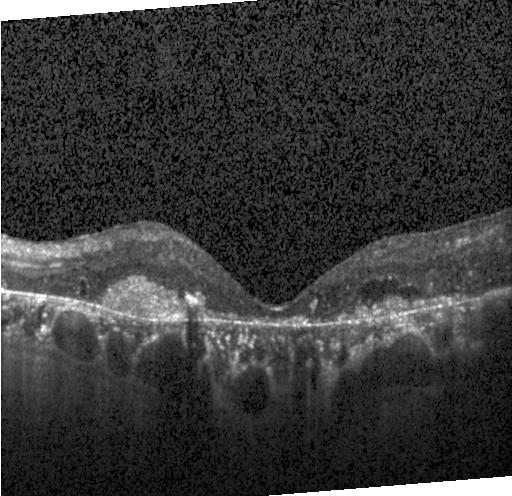
OCT finding: a choroidal neovascular membrane.